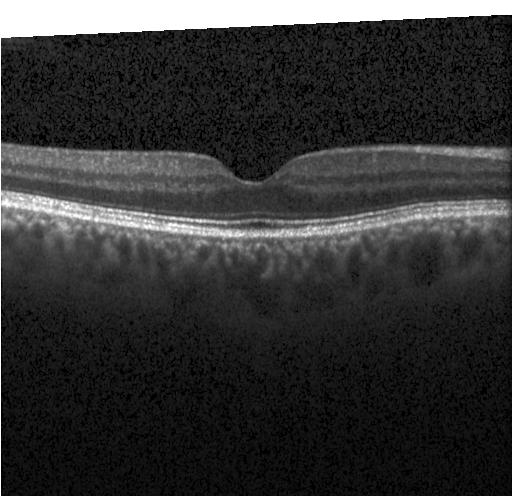 Spectral-domain optical coherence tomography; OCT line scan; acquired on a Heidelberg Spectralis. Dx: no evidence of CNV, DME, or drusen.